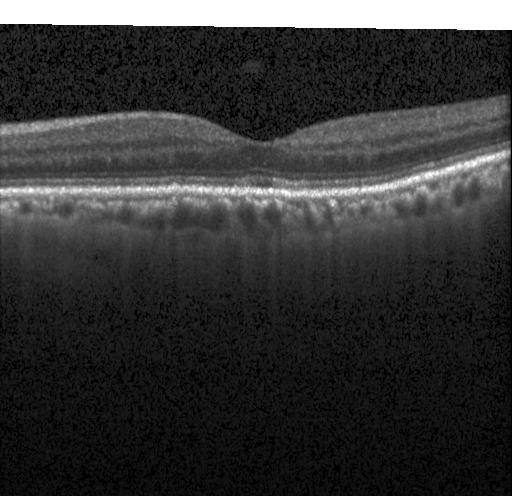

Retinal OCT cross-section · macular scan
Diagnosis: neither choroidal neovascularization, diabetic macular edema, nor drusen.